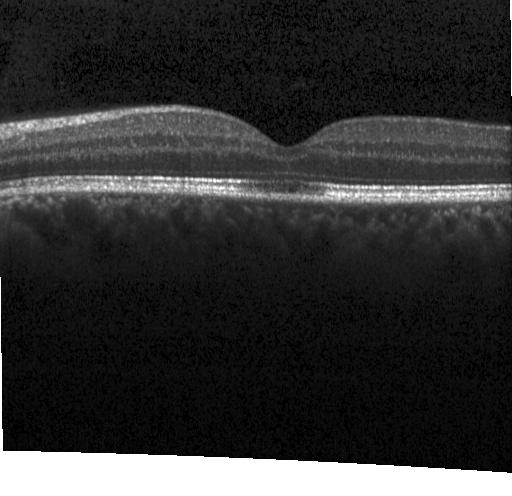 Acquired on a Heidelberg Spectralis. SD-OCT. OCT B-scan — No evidence of CNV, DME, or drusen.